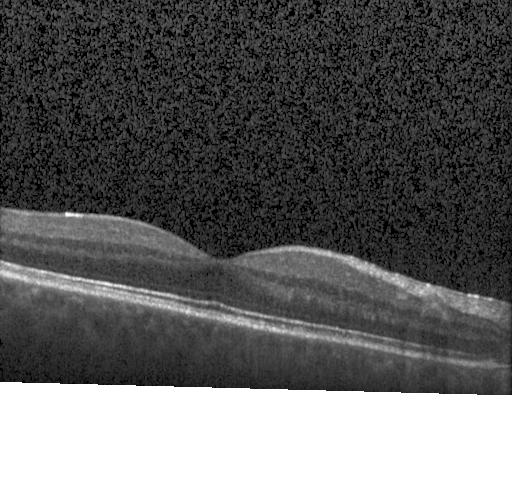

Diagnosis: no CNV, no DME, and no drusen.